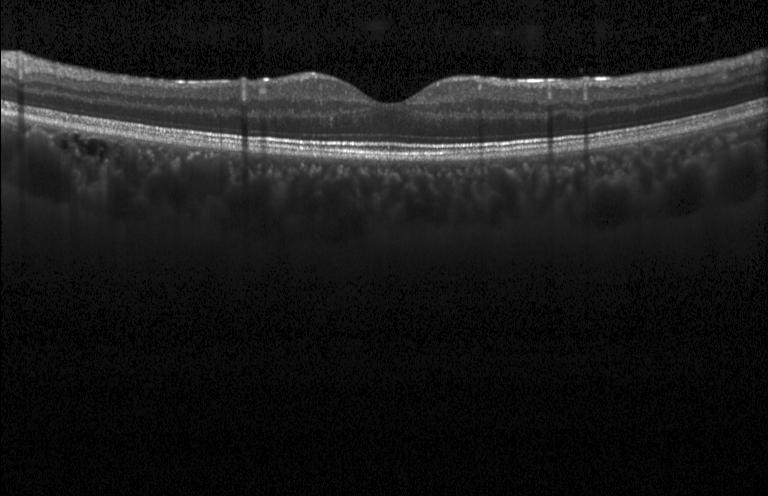
OCT B-scan. Diagnosis: neither choroidal neovascularization, diabetic macular edema, nor drusen.